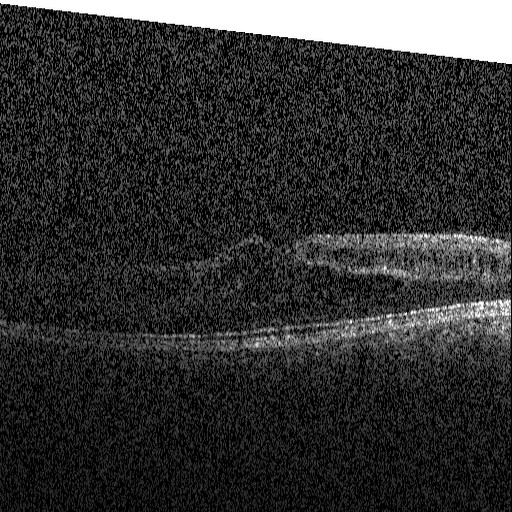

Macular scan, OCT B-scan, instrument: Heidelberg Spectralis — Macular OCT: DME.